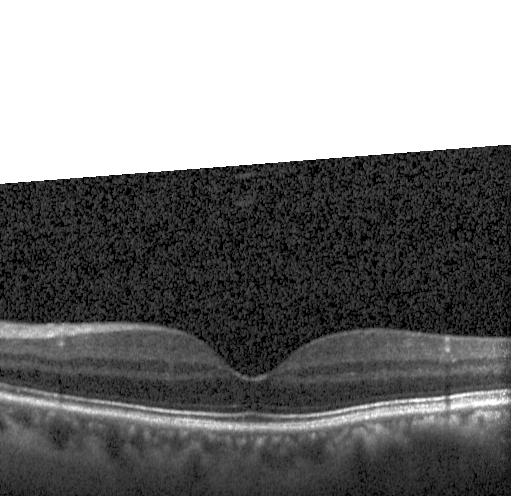 Optical coherence tomography B-scan. Macular OCT: no CNV, DME, or drusen.